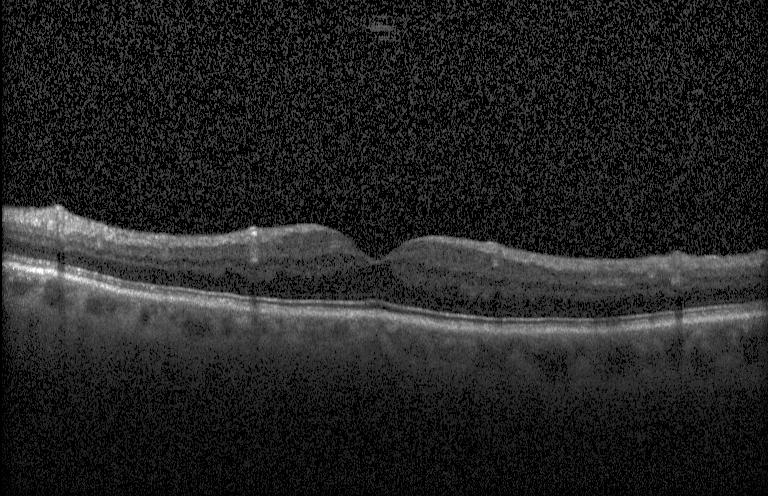 OCT line scan, centered on the fovea, SD-OCT, Heidelberg Spectralis OCT system.
Neither choroidal neovascularization, diabetic macular edema, nor drusen.